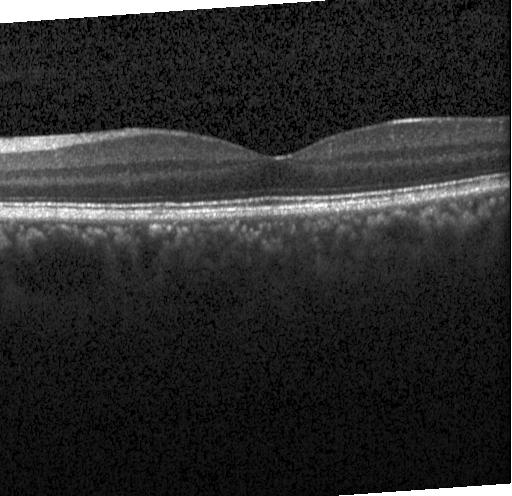 Diagnosis: no CNV, no DME, and no drusen.